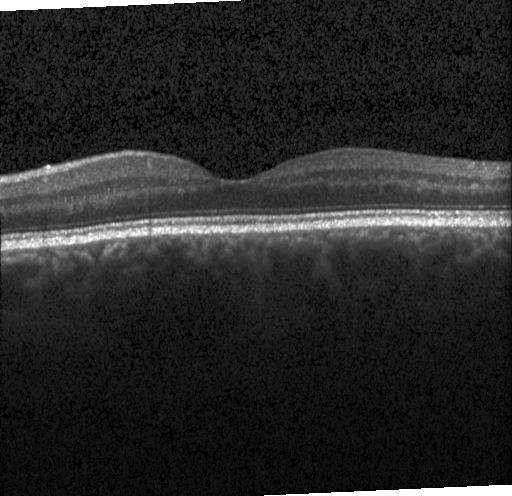
Optical coherence tomography B-scan. Acquired on a Heidelberg Spectralis — Dx: no CNV, DME, or drusen.